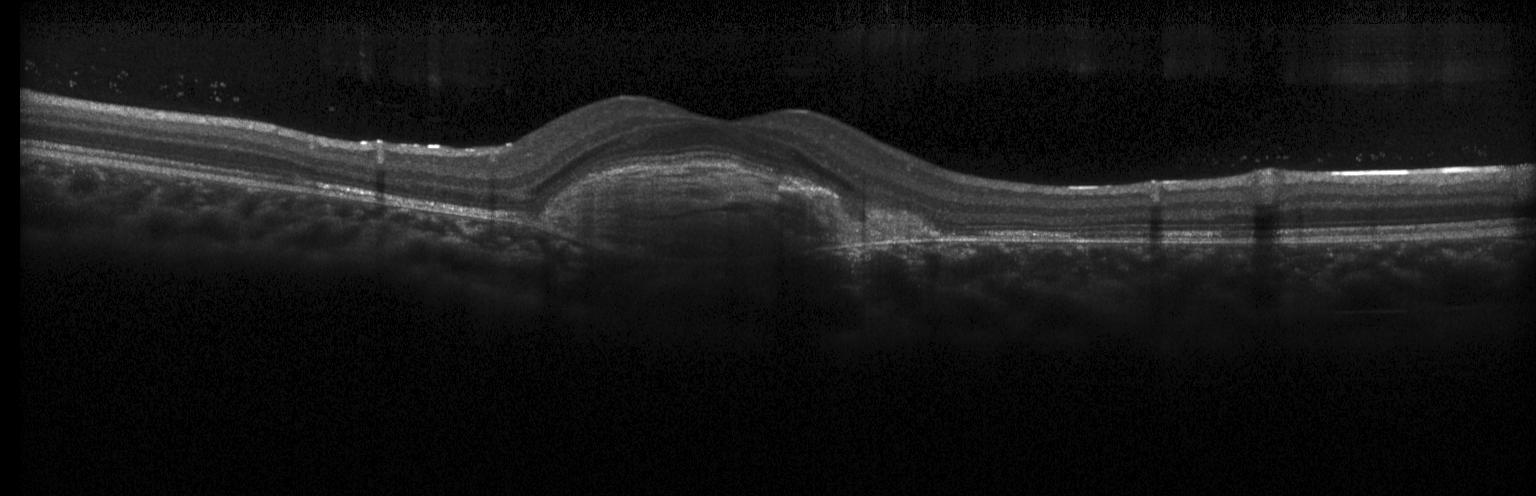 OCT line scan; Heidelberg Spectralis OCT system.
Impression: a choroidal neovascular membrane.